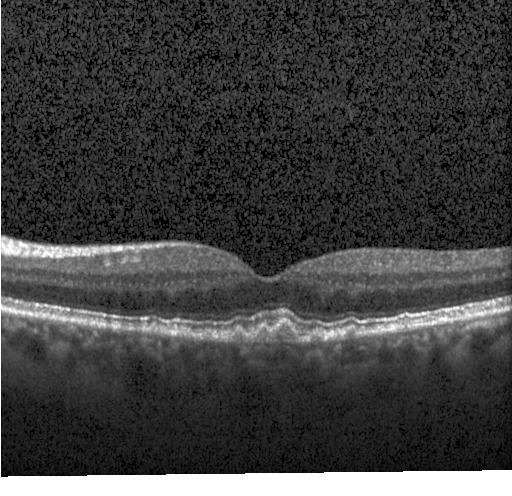
Retinal OCT cross-section; macular scan. Diagnosis: sub-RPE drusenoid deposits.